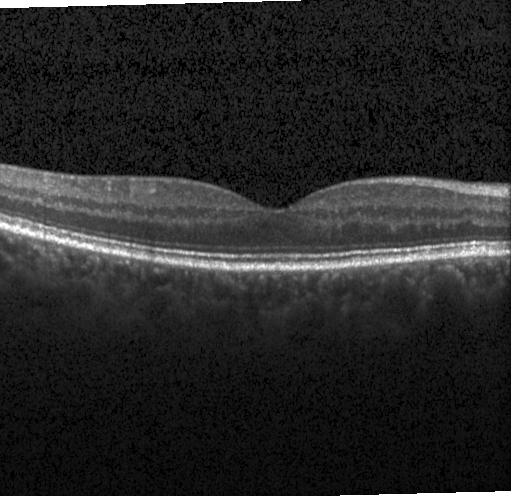 OCT line scan. Horizontal scan through the fovea. Heidelberg Spectralis OCT system
Macular OCT: no CNV, DME, or drusen.